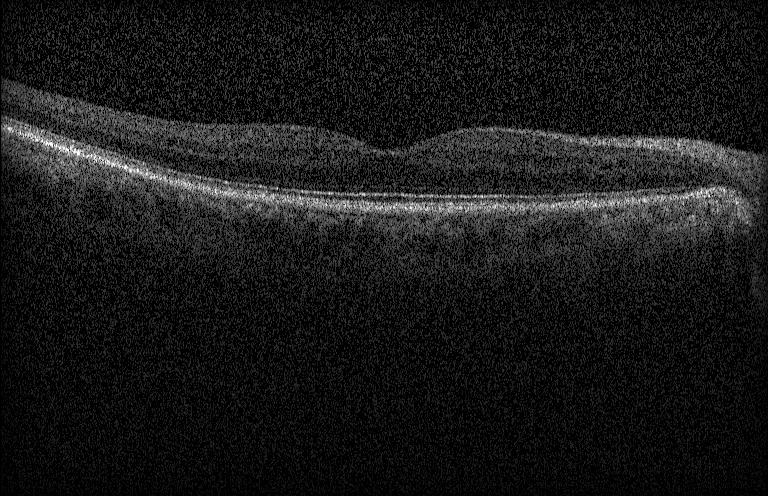 Spectral-domain OCT. Optical coherence tomography scan. Heidelberg Spectralis OCT system. Centered on the fovea.
Finding: no evidence of choroidal neovascularization, diabetic macular edema, or drusen.